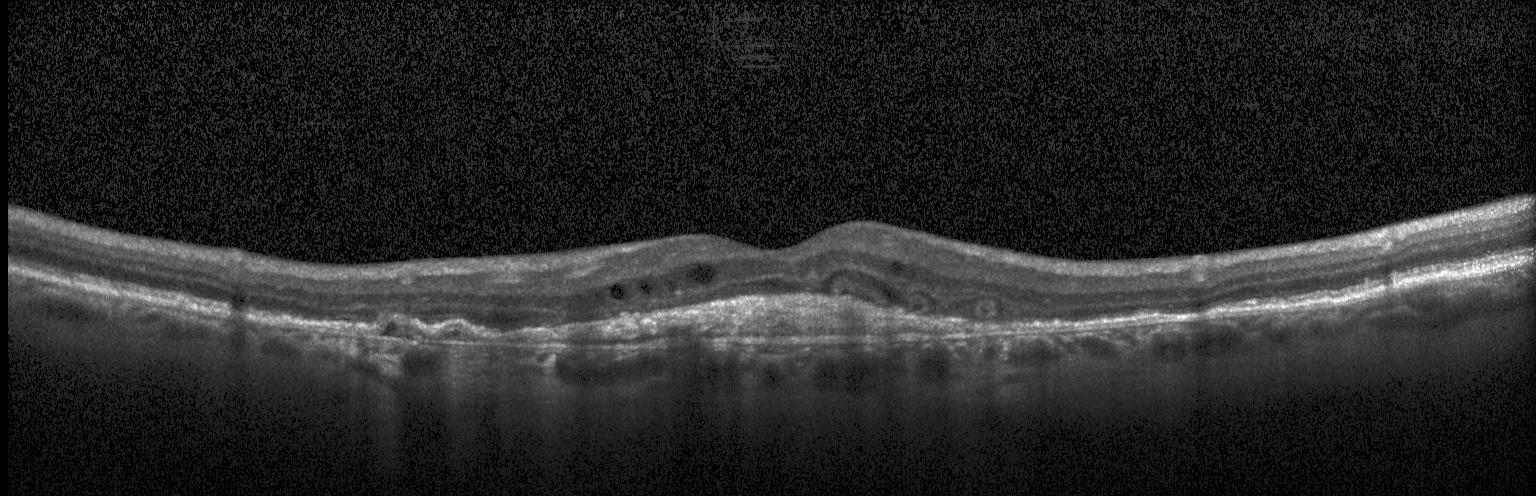
Retinal OCT B-scan, SD-OCT — OCT finding: choroidal neovascularization (CNV).